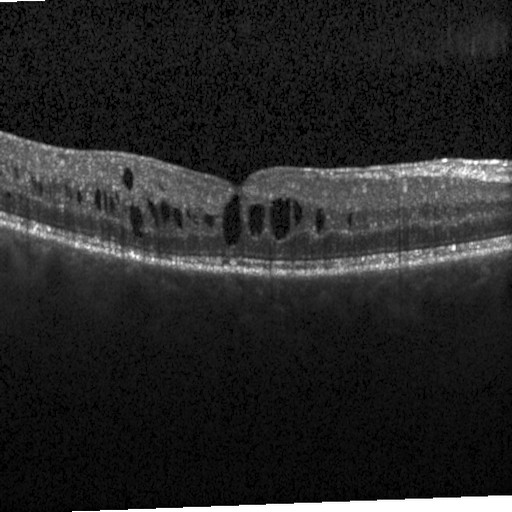

Heidelberg Spectralis, horizontal scan through the fovea, spectral-domain OCT, retinal OCT B-scan. Finding: diabetic macular edema (DME).